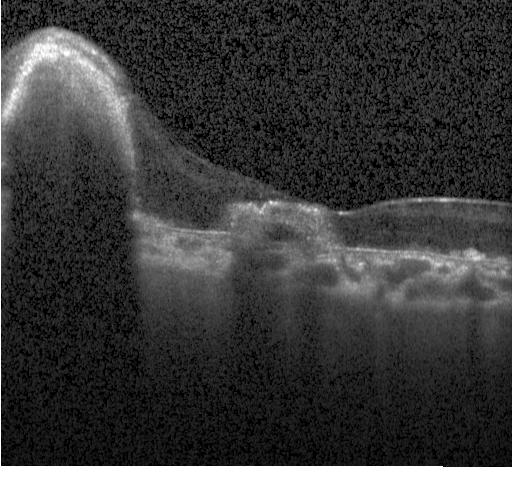 Fovea-centered; optical coherence tomography B-scan; instrument: Heidelberg Spectralis; spectral-domain OCT. Diagnosis: CNV.